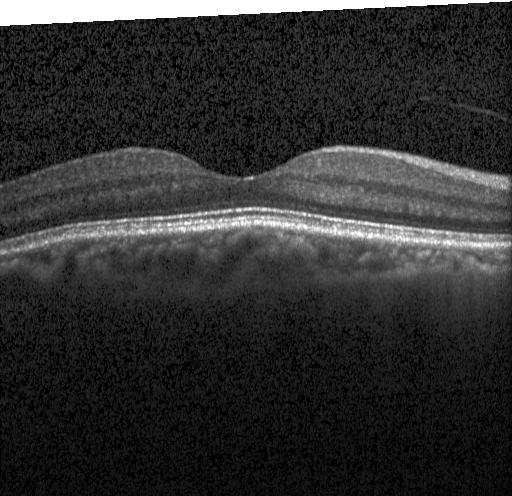
Optical coherence tomography scan, fovea-centered — Macular OCT: no CNV, DME, or drusen.